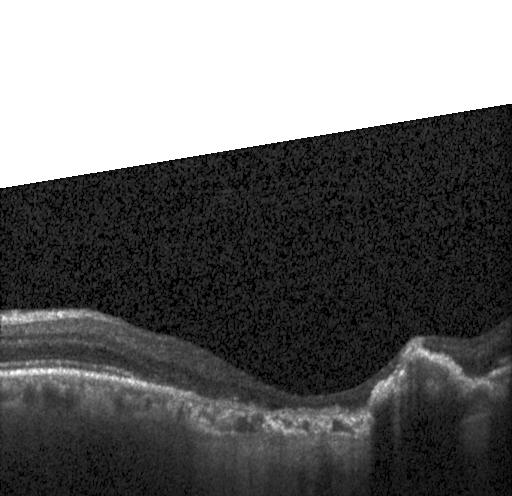

Impression: choroidal neovascularization (CNV).